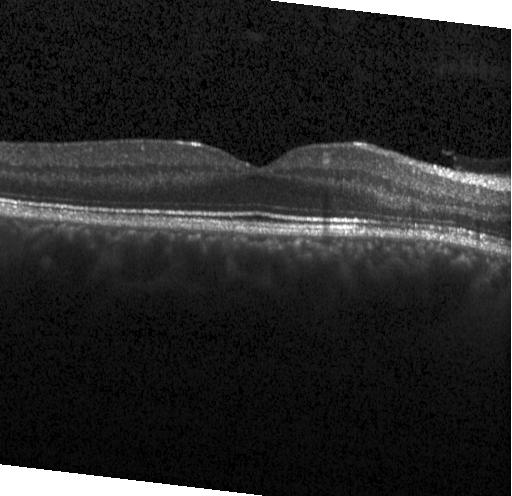

OCT line scan; horizontal scan through the fovea; acquired on a Heidelberg Spectralis — Neither CNV, DME, nor drusen.